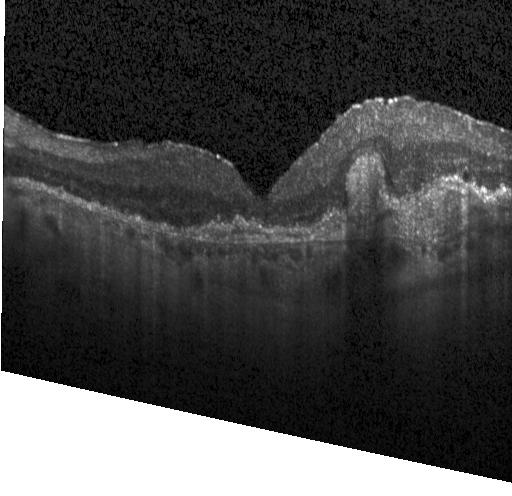
Optical coherence tomography B-scan.
Dx: a choroidal neovascular membrane.